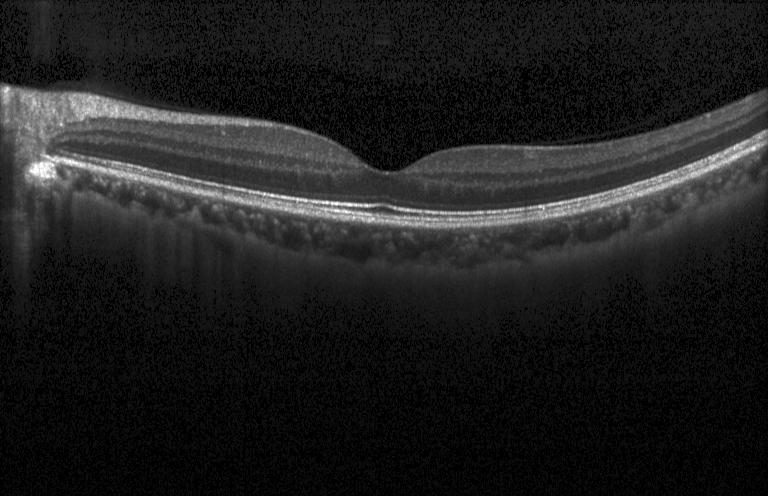 Heidelberg Spectralis; optical coherence tomography B-scan.
Diagnosis: neither CNV, DME, nor drusen.